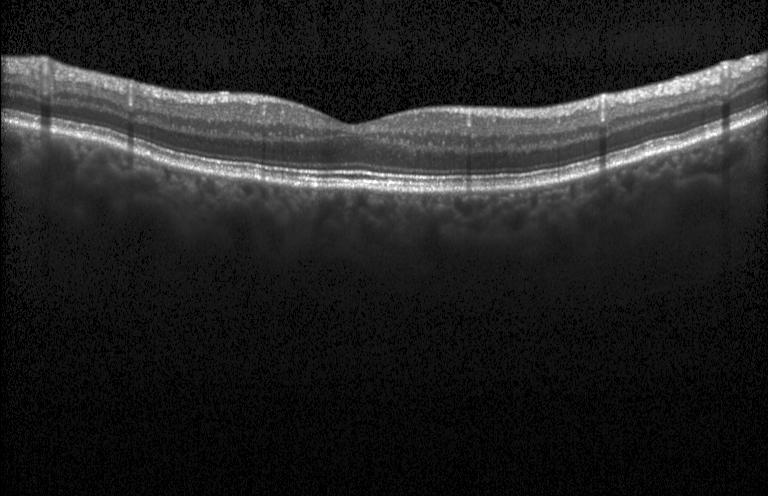 This B-scan demonstrates no evidence of choroidal neovascularization, diabetic macular edema, or drusen.